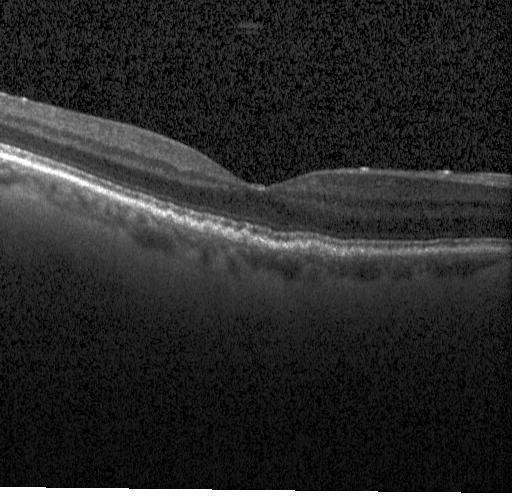
Heidelberg Spectralis · through the macula · retinal OCT B-scan.
Drusen.